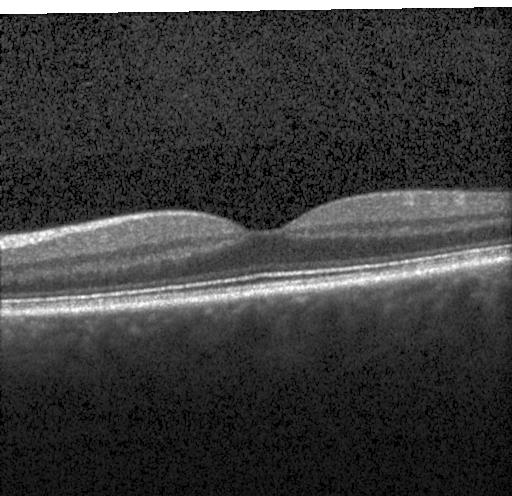 OCT scan showing no evidence of CNV, DME, or drusen.